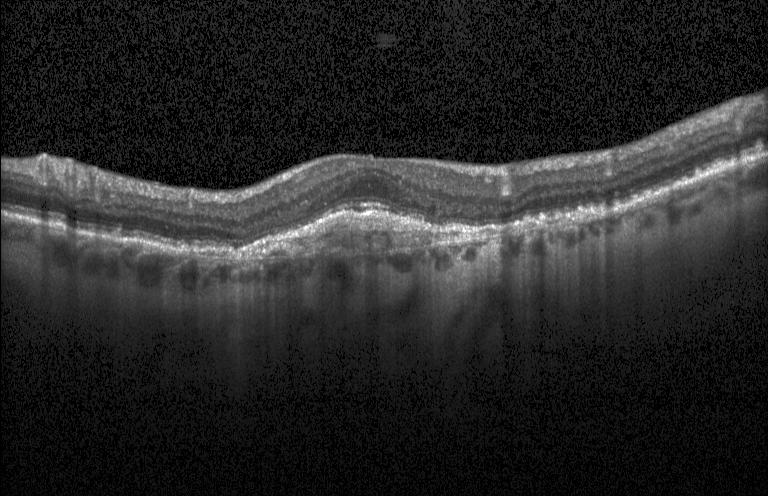

Dx: CNV.